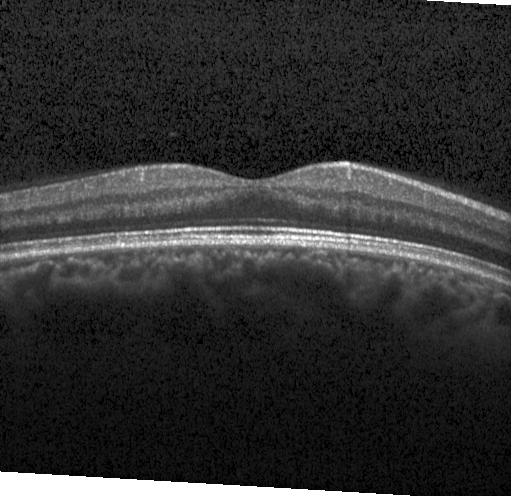
Macular OCT demonstrating no evidence of CNV, DME, or drusen.